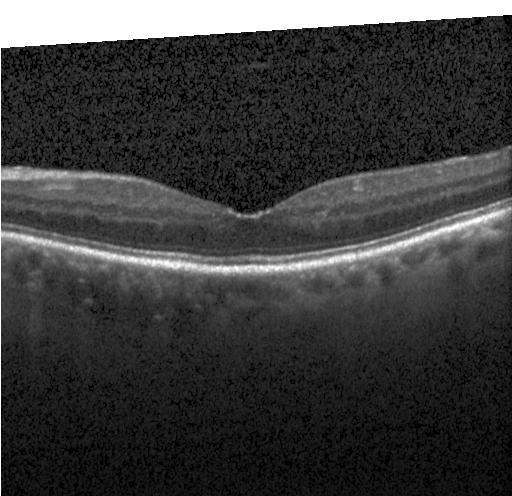 Macular OCT: neither CNV, DME, nor drusen.